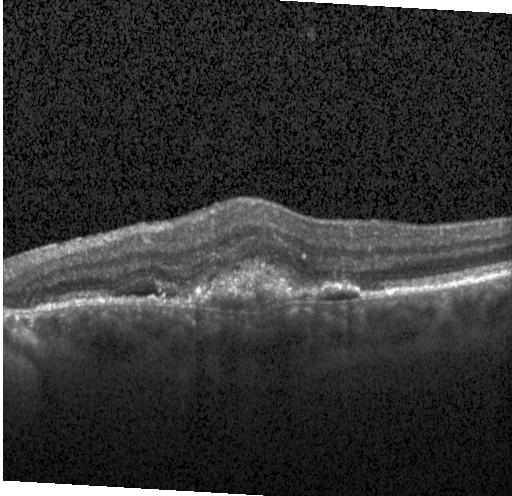
This B-scan demonstrates choroidal neovascularization (CNV).